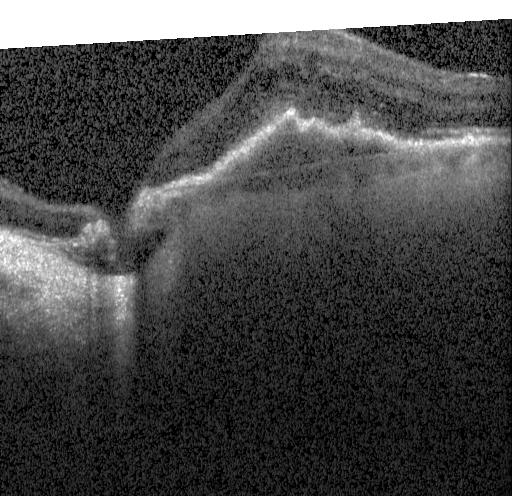

OCT B-scan, centered on the fovea
Choroidal neovascularization (CNV).